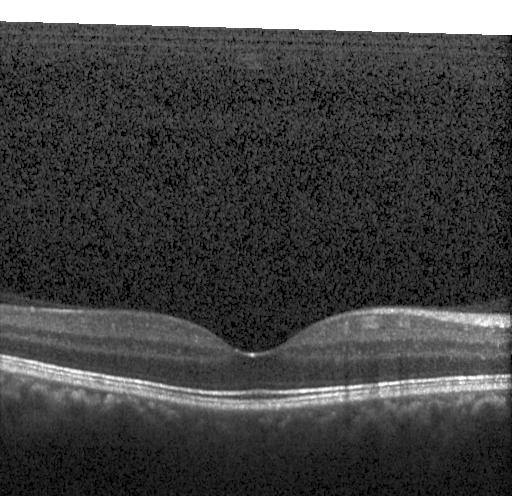 SD-OCT · through the macula · retinal OCT B-scan · Heidelberg Spectralis OCT system. Finding: no choroidal neovascularization, diabetic macular edema, or drusen.